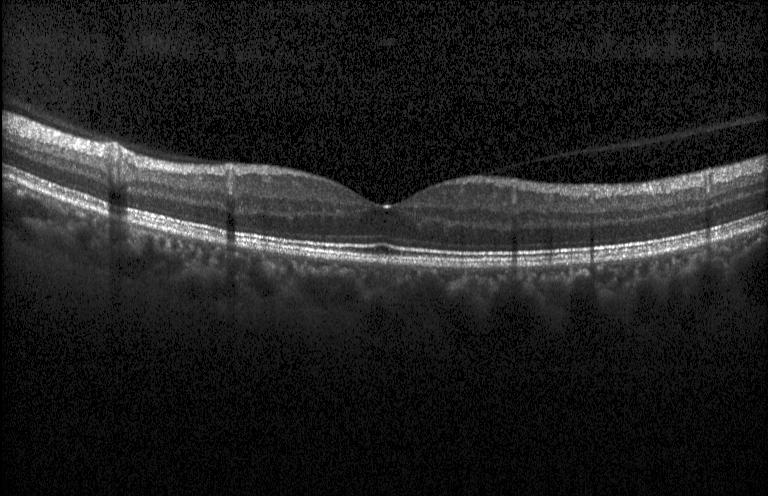 OCT finding: no choroidal neovascularization, no diabetic macular edema, and no drusen.